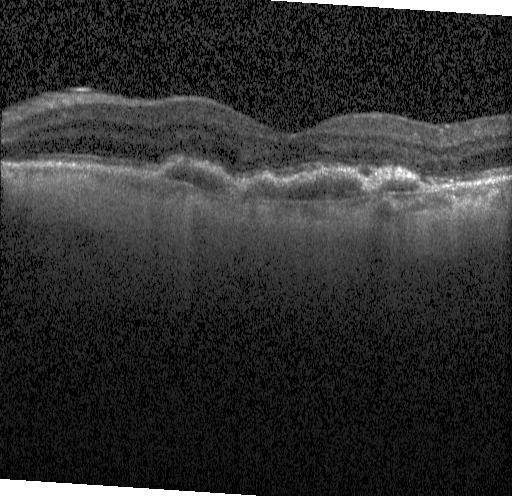
Retinal OCT B-scan — Macular OCT: a choroidal neovascular membrane.